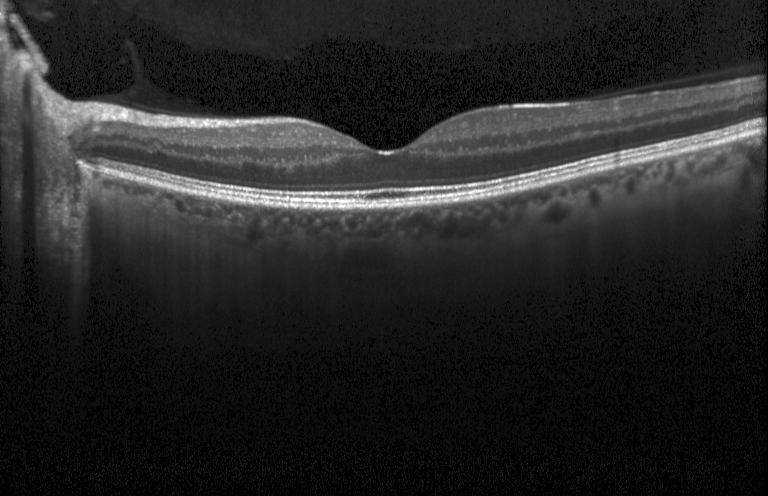 Macular OCT: no evidence of choroidal neovascularization, diabetic macular edema, or drusen.